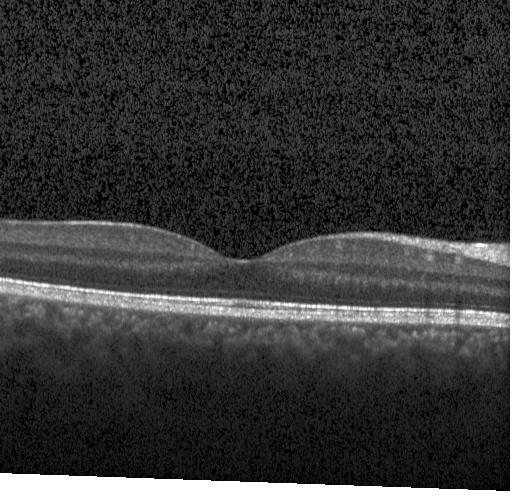

Dx: neither CNV, DME, nor drusen.